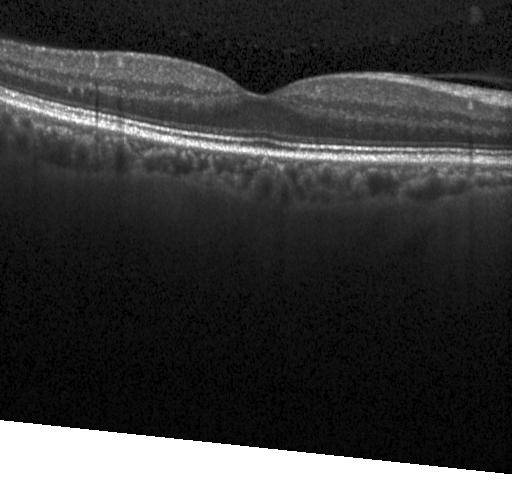

The scan shows no evidence of choroidal neovascularization, diabetic macular edema, or drusen.